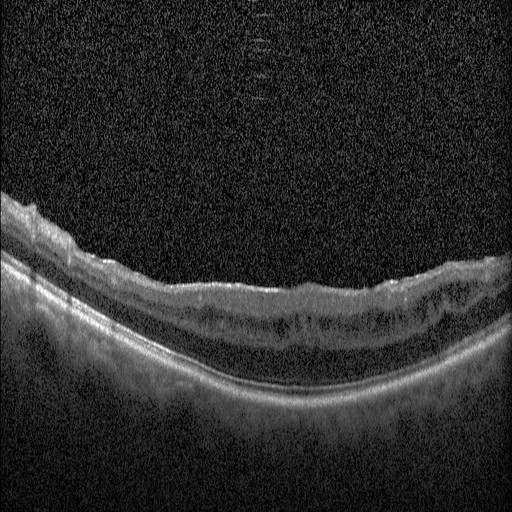

Spectral-domain OCT; OCT B-scan; horizontal scan through the fovea; Heidelberg Spectralis OCT system.
Impression: DME.